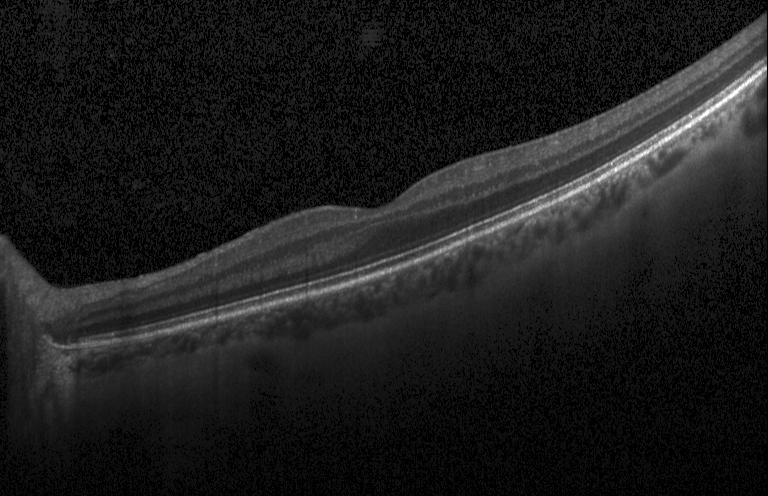

Spectral-domain OCT B-scan: no CNV, no DME, and no drusen.